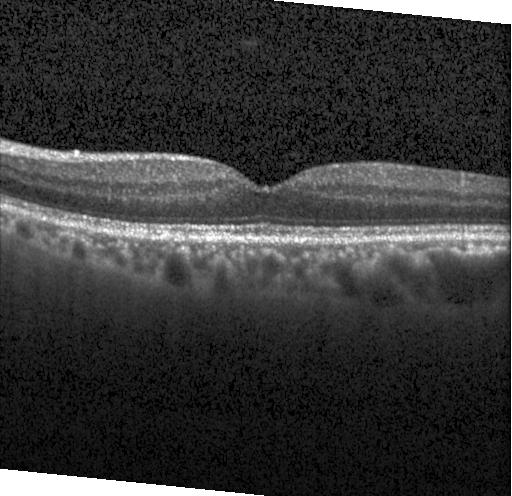 OCT B-scan showing no choroidal neovascularization, no diabetic macular edema, and no drusen.